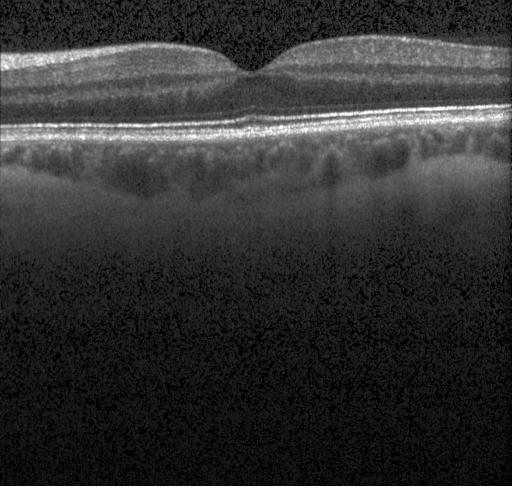 Retinal OCT cross-section — Finding: no evidence of CNV, DME, or drusen.